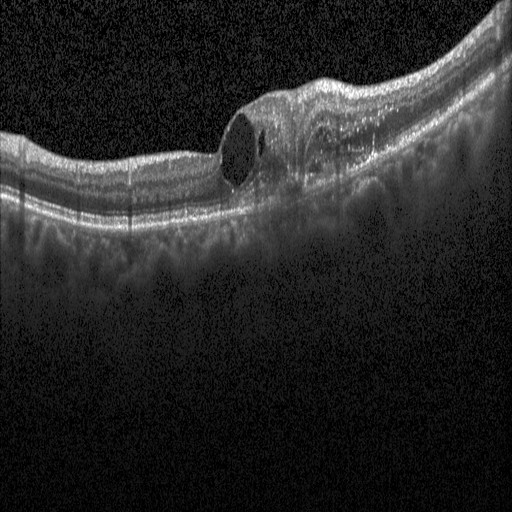
Retinal OCT cross-section. Spectral-domain optical coherence tomography — Diagnosis: DME.